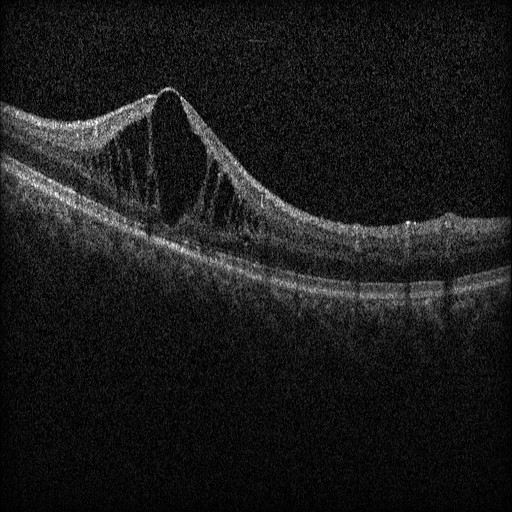
Retinal OCT B-scan.
Assessment: DME.